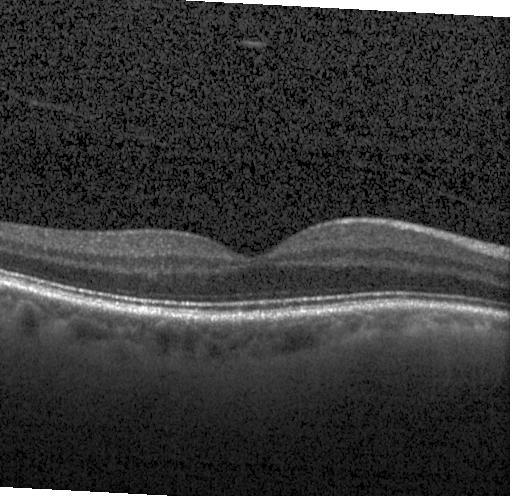
OCT line scan. Acquired on a Heidelberg Spectralis. SD-OCT. Fovea-centered. Diagnosis: no CNV, DME, or drusen.